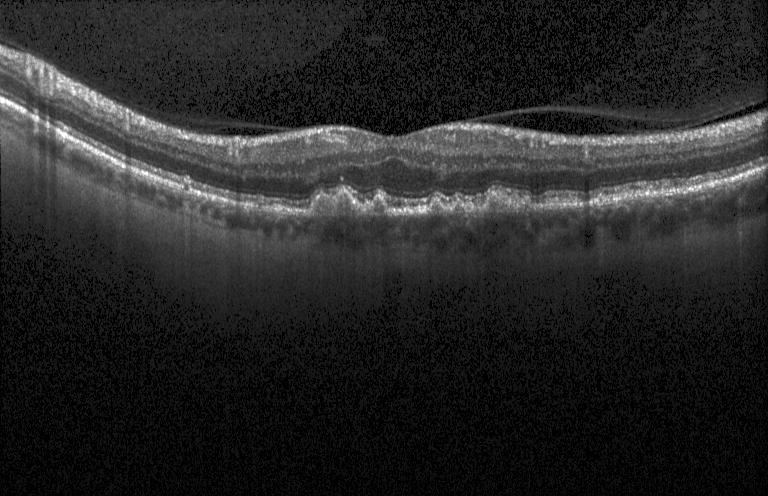
Retinal OCT cross-section, acquired on a Heidelberg Spectralis
Assessment: drusen.